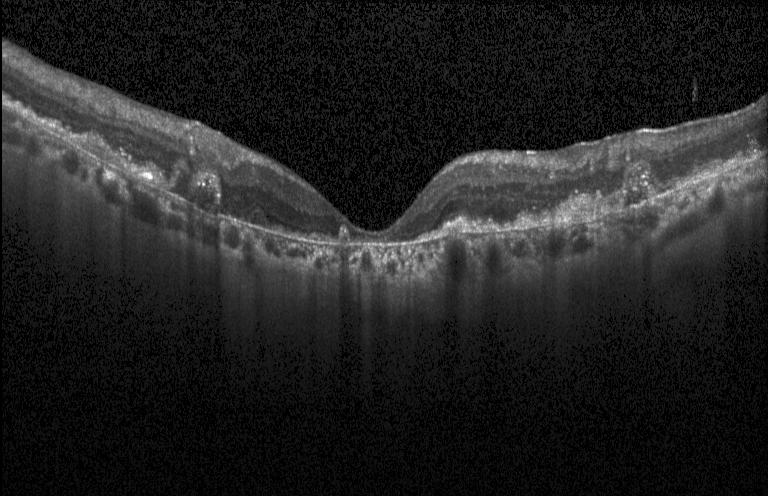
Dx: CNV.